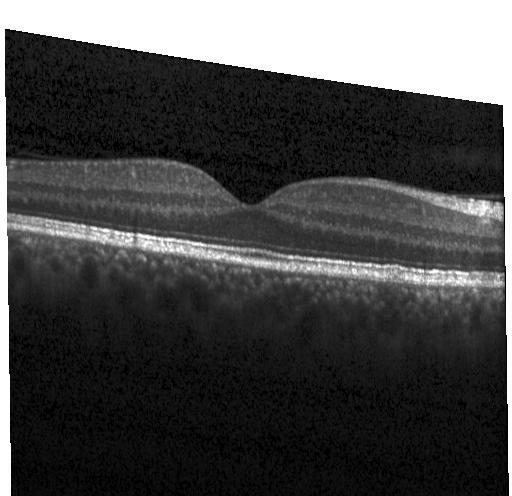 Optical coherence tomography scan
Impression: no evidence of choroidal neovascularization, diabetic macular edema, or drusen.